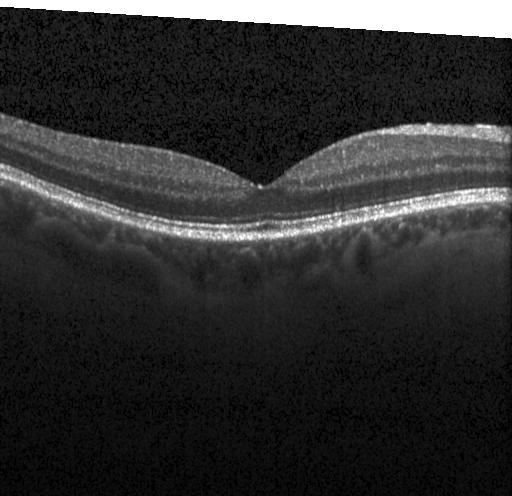

OCT finding: no evidence of CNV, DME, or drusen.